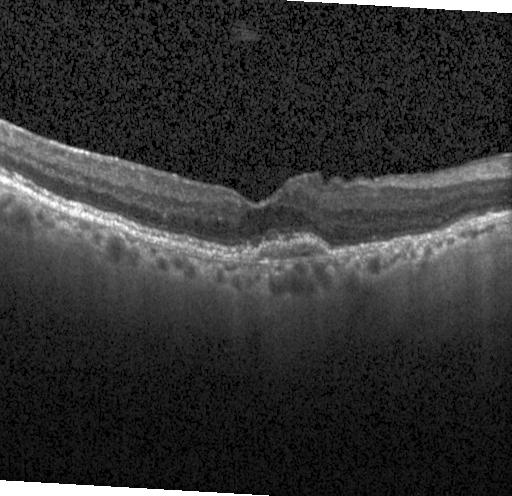

Retinal OCT cross-section · acquired on a Heidelberg Spectralis · centered on the fovea · SD-OCT — Impression: a choroidal neovascular membrane.